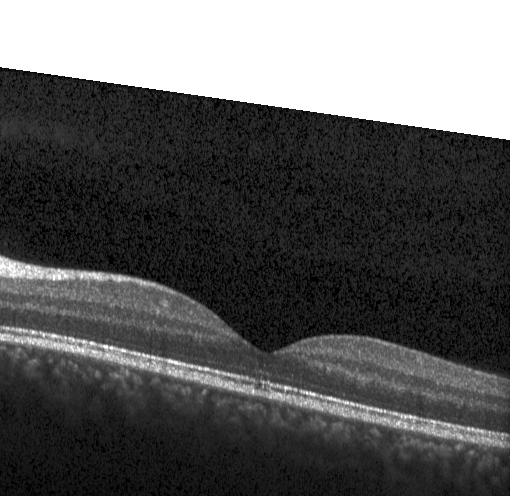

Retinal OCT cross-section showing no choroidal neovascularization, diabetic macular edema, or drusen.